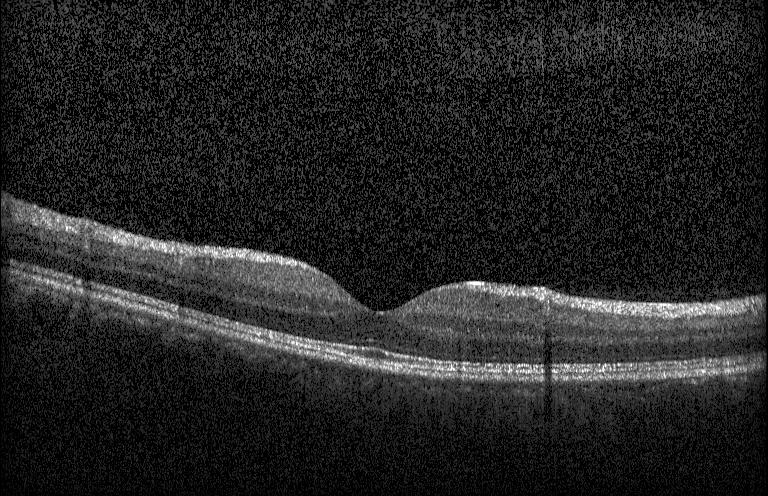

OCT scan showing neither CNV, DME, nor drusen.